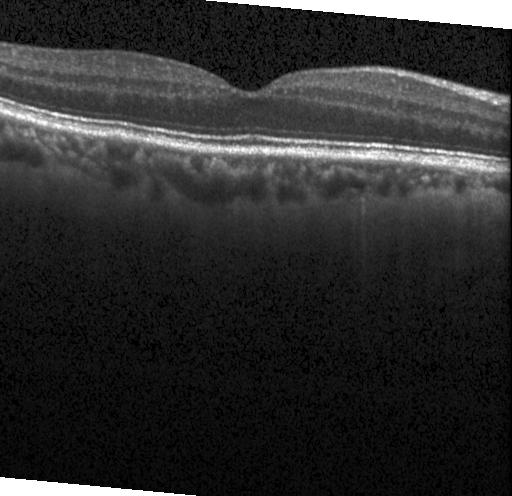

Heidelberg Spectralis OCT system · retinal OCT cross-section. Assessment: no choroidal neovascularization, diabetic macular edema, or drusen.